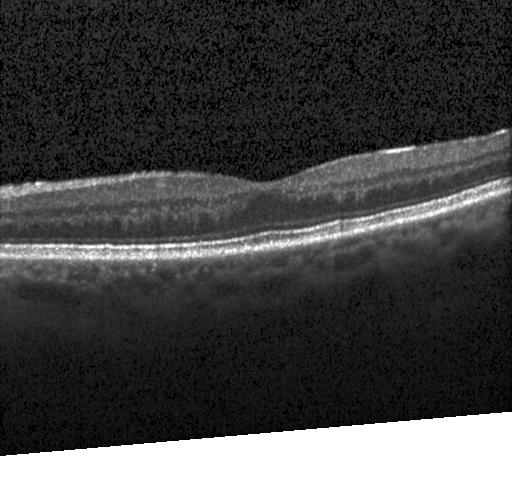

Horizontal scan through the fovea, SD-OCT, optical coherence tomography scan.
Assessment: no CNV, DME, or drusen.